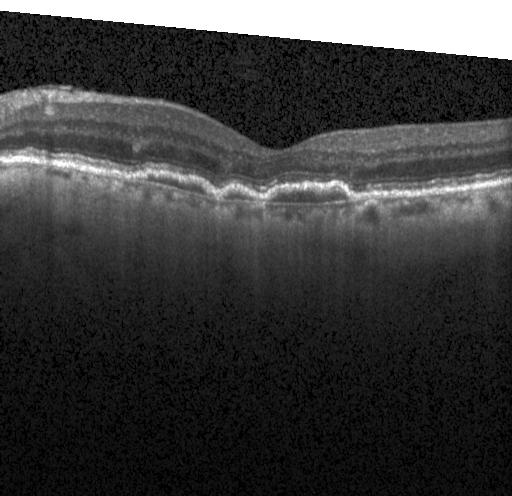 Diagnosis: a choroidal neovascular membrane.